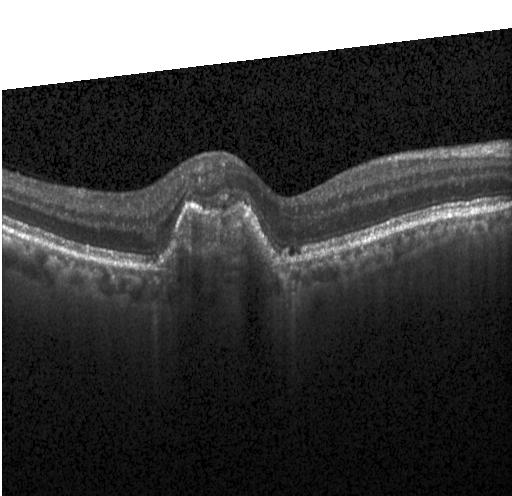
Instrument: Heidelberg Spectralis, OCT B-scan, through the macula.
Finding: a choroidal neovascular membrane.